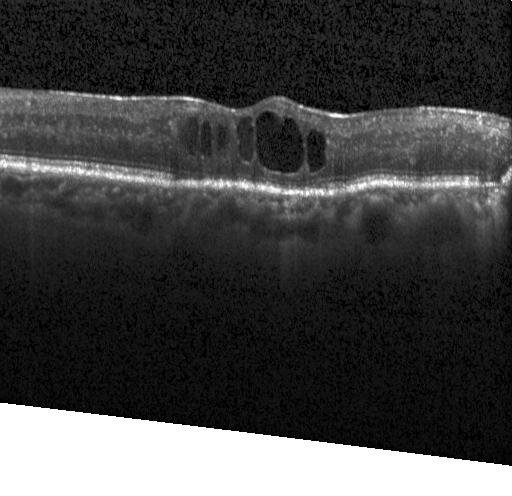

Retinal OCT B-scan. Spectral-domain OCT. Macular scan. Acquired on a Heidelberg Spectralis. Diagnosis: DME.